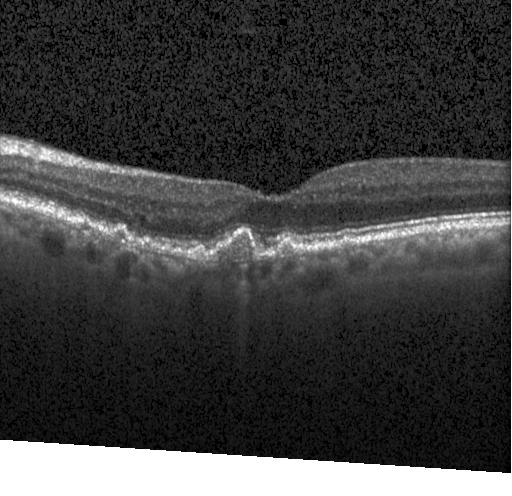

Dx: sub-RPE drusenoid deposits.